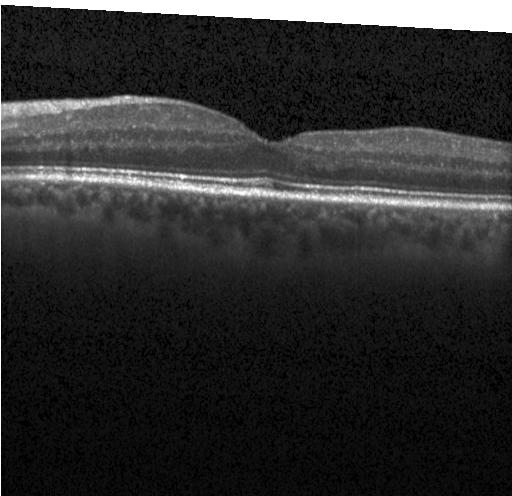
Horizontal scan through the fovea. Retinal OCT cross-section. Heidelberg Spectralis. SD-OCT. Finding: no choroidal neovascularization, diabetic macular edema, or drusen.